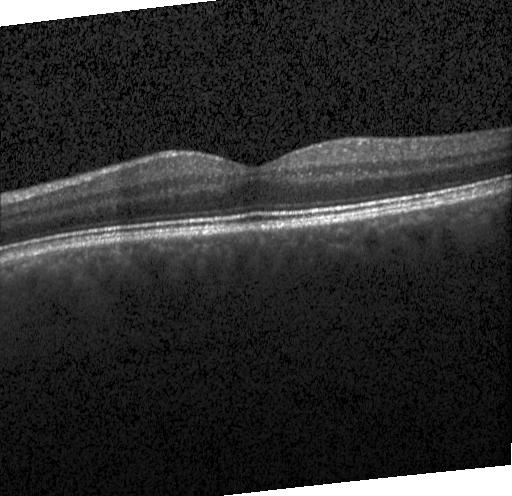

Retinal OCT B-scan. Diagnosis: no CNV, DME, or drusen.